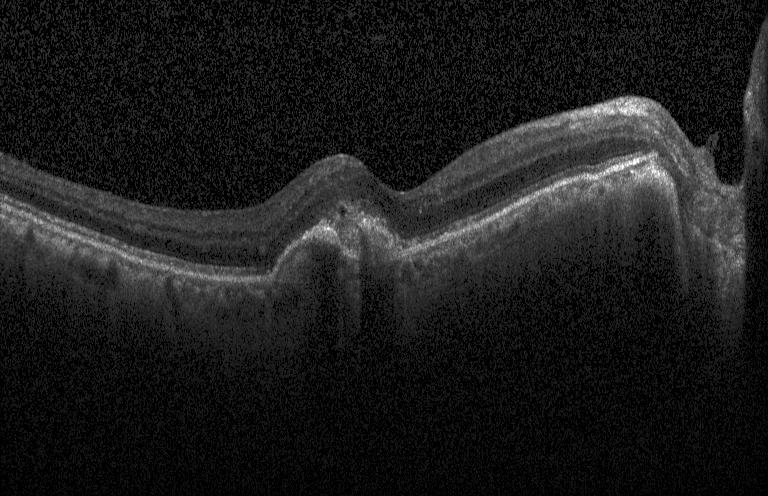

Spectral-domain optical coherence tomography. Optical coherence tomography scan. Finding: a choroidal neovascular membrane.